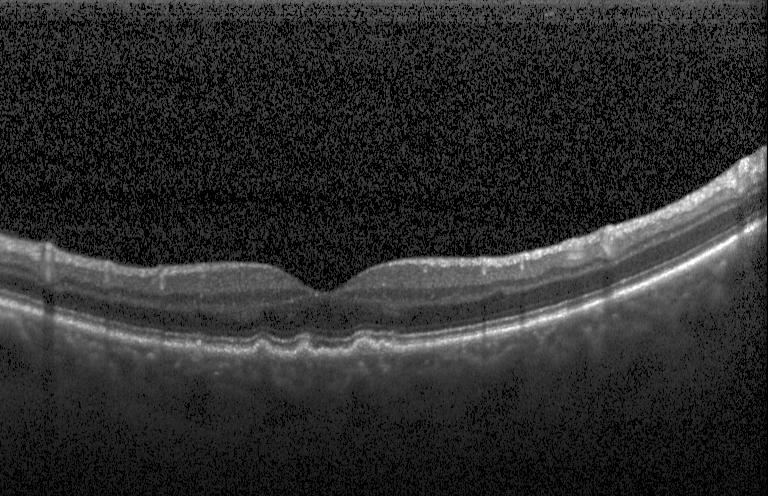

Retinal OCT B-scan · instrument: Heidelberg Spectralis · through the macula — Impression: sub-RPE drusenoid deposits.